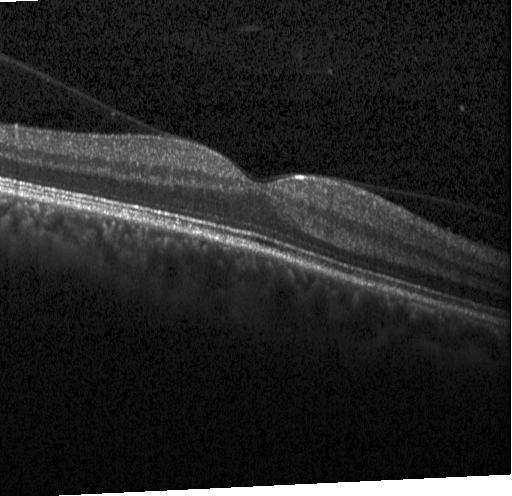
Optical coherence tomography scan; acquired on a Heidelberg Spectralis.
Assessment: no choroidal neovascularization, diabetic macular edema, or drusen.